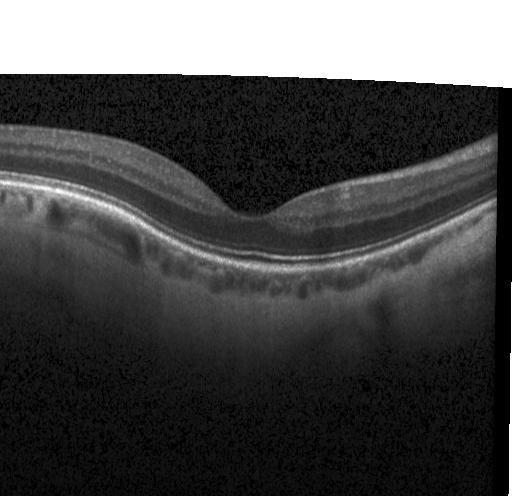

Finding: no choroidal neovascularization, no diabetic macular edema, and no drusen.